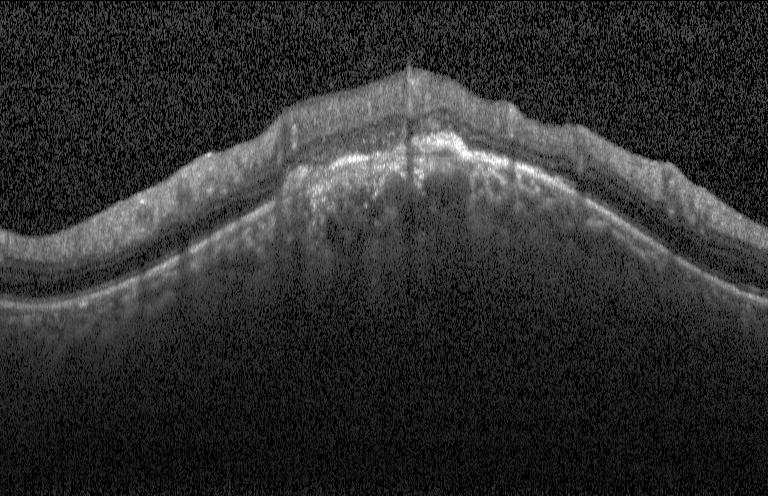
Fovea-centered. Optical coherence tomography B-scan — Macular OCT: choroidal neovascularization.